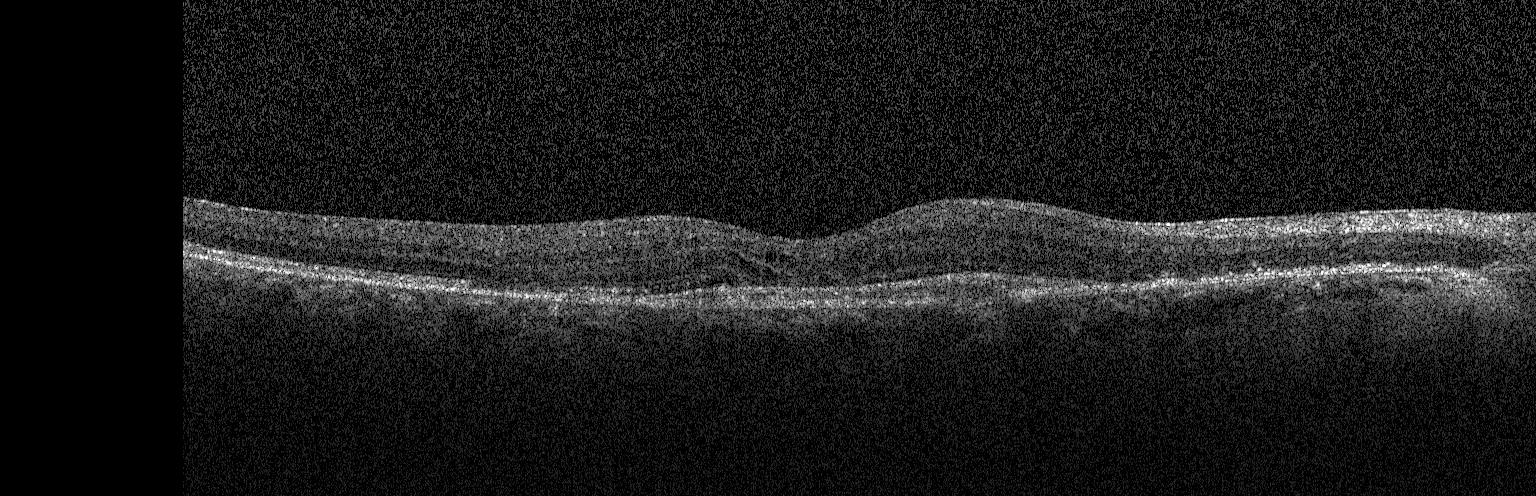

Instrument: Heidelberg Spectralis · retinal OCT cross-section · spectral-domain OCT · horizontal scan through the fovea. Macular OCT: CNV.